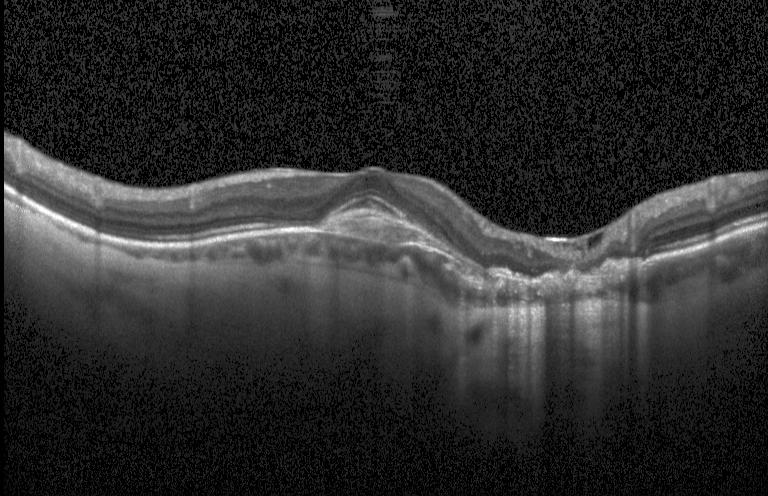

Spectral-domain OCT B-scan: a choroidal neovascular membrane.